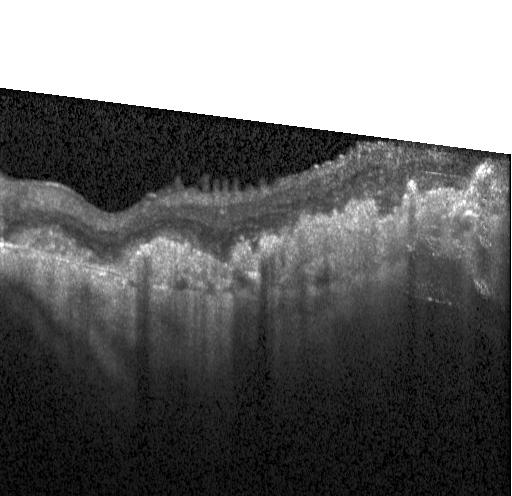

Dx: a choroidal neovascular membrane.